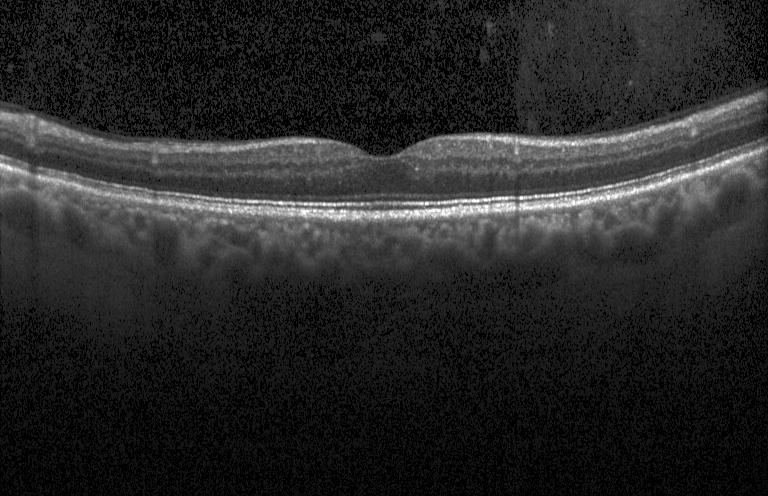 Spectral-domain optical coherence tomography · Heidelberg Spectralis · optical coherence tomography scan. This B-scan demonstrates no choroidal neovascularization, diabetic macular edema, or drusen.